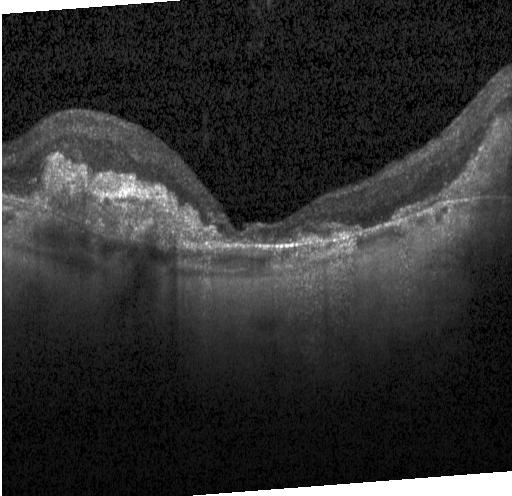
Acquired on a Heidelberg Spectralis · spectral-domain optical coherence tomography · fovea-centered · optical coherence tomography scan. Assessment: choroidal neovascularization.